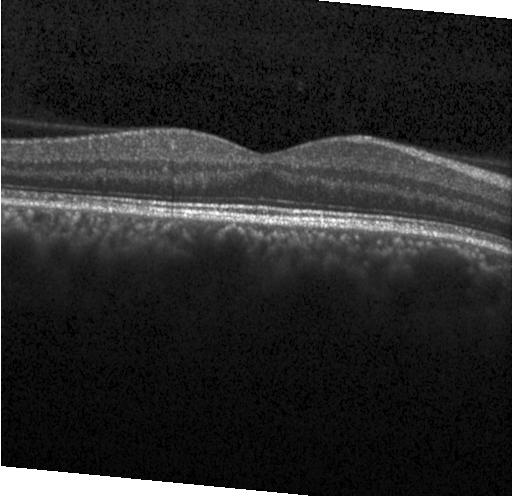 Optical coherence tomography scan; SD-OCT; fovea-centered; acquired on a Heidelberg Spectralis. The scan shows no evidence of choroidal neovascularization, diabetic macular edema, or drusen.